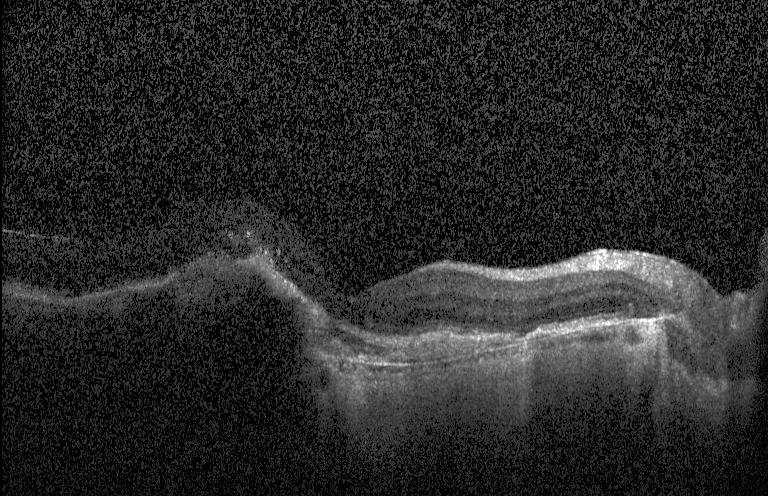
This B-scan demonstrates a choroidal neovascular membrane.